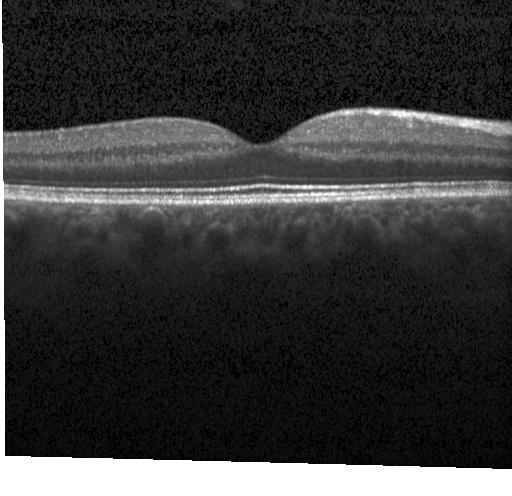

OCT B-scan showing neither choroidal neovascularization, diabetic macular edema, nor drusen.